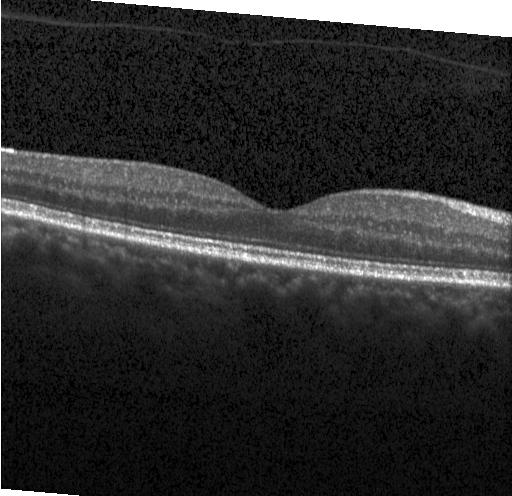
OCT scan showing no CNV, no DME, and no drusen.